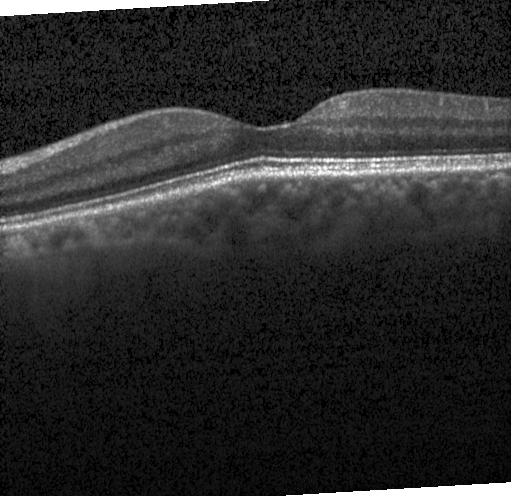
Diagnosis: no evidence of choroidal neovascularization, diabetic macular edema, or drusen.